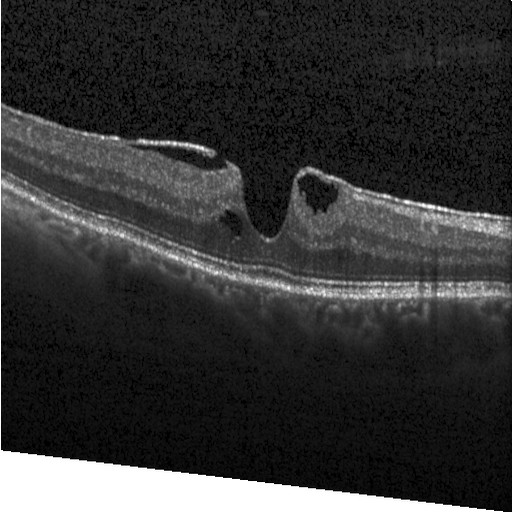
OCT B-scan — This B-scan demonstrates diabetic macular edema.